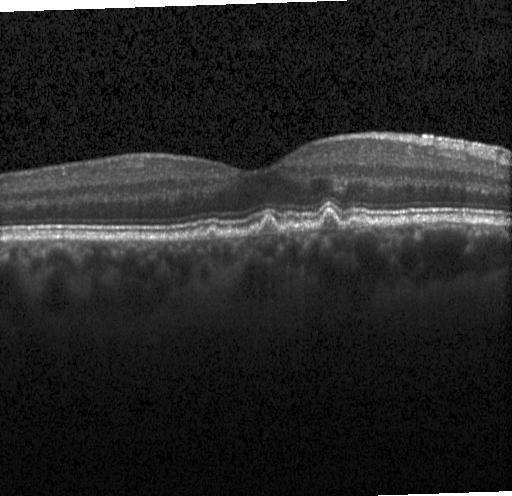

OCT B-scan · spectral-domain OCT. Drusen.